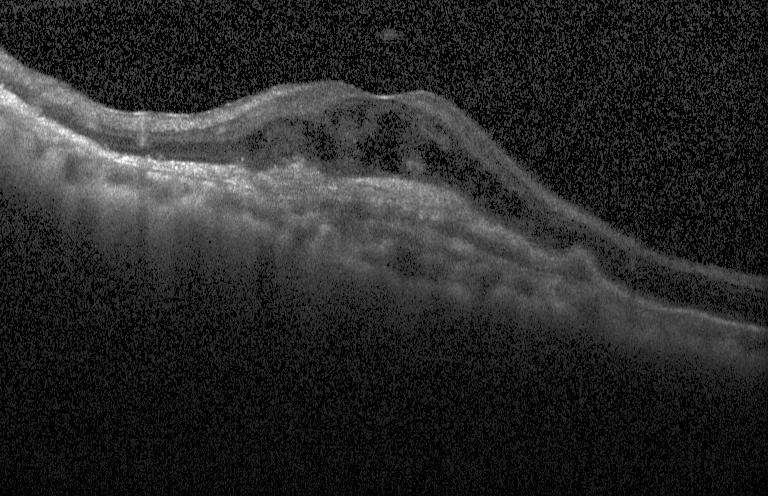 Centered on the fovea, OCT line scan.
Assessment: a choroidal neovascular membrane.